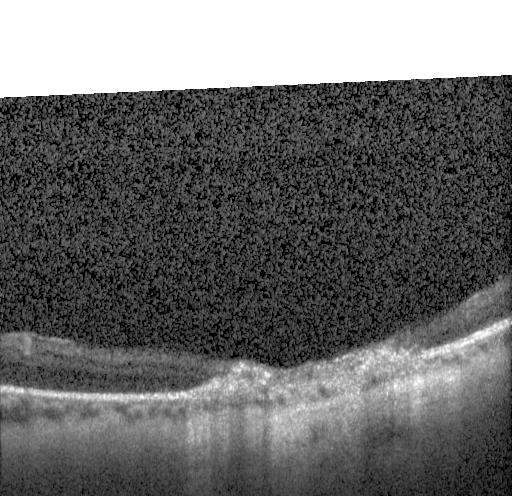
Finding: a choroidal neovascular membrane.